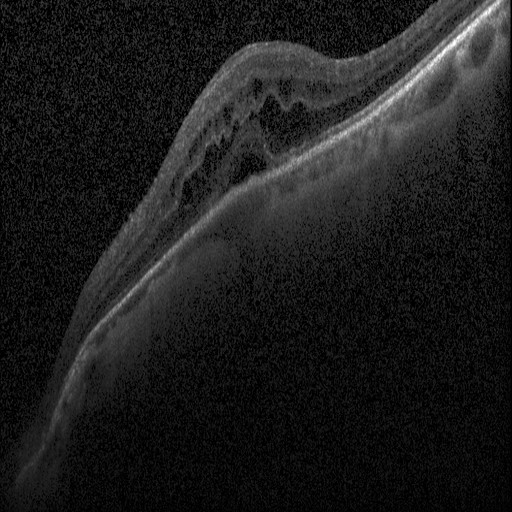 Centered on the fovea. Optical coherence tomography scan. Heidelberg Spectralis
Diagnosis: DME.